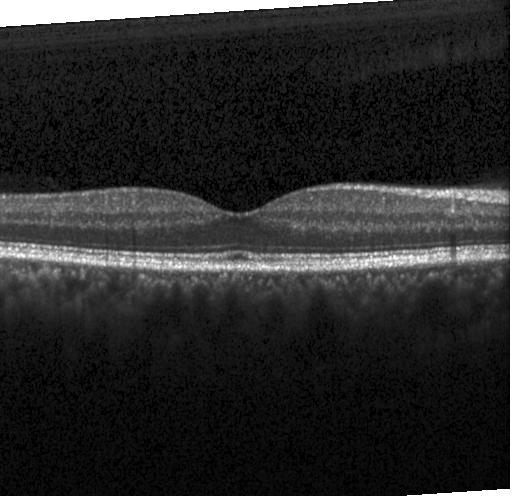
This B-scan demonstrates no CNV, no DME, and no drusen.